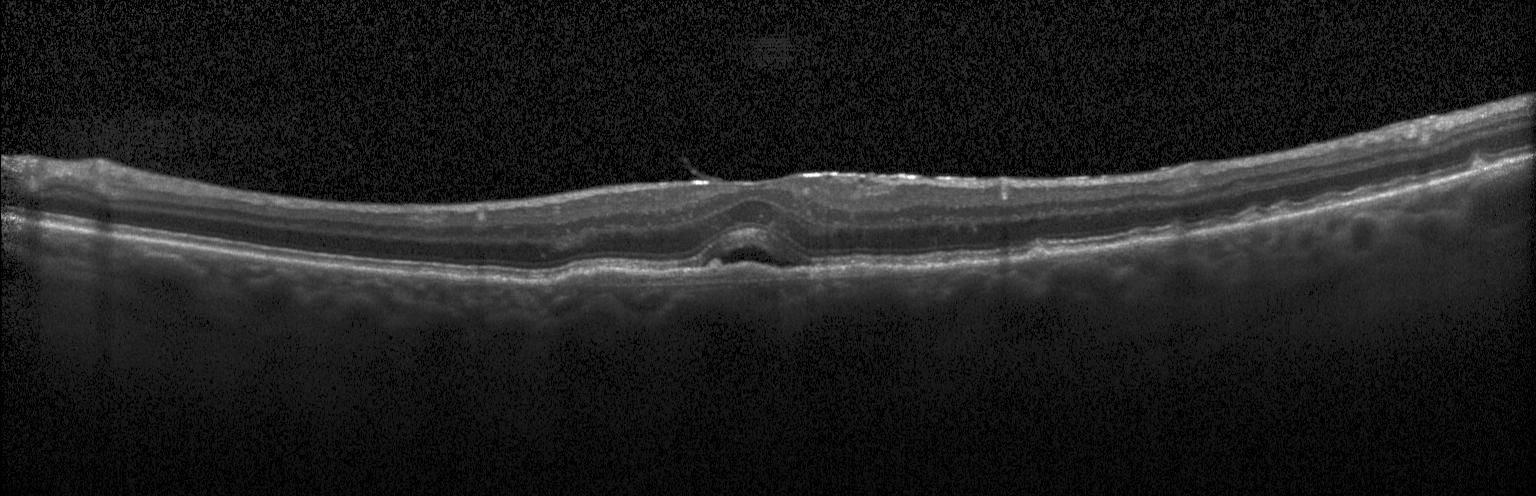 Optical coherence tomography scan · centered on the fovea — Impression: choroidal neovascularization.